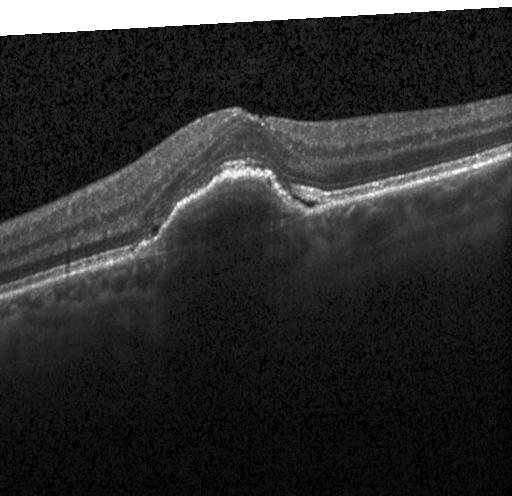 The scan shows a choroidal neovascular membrane.